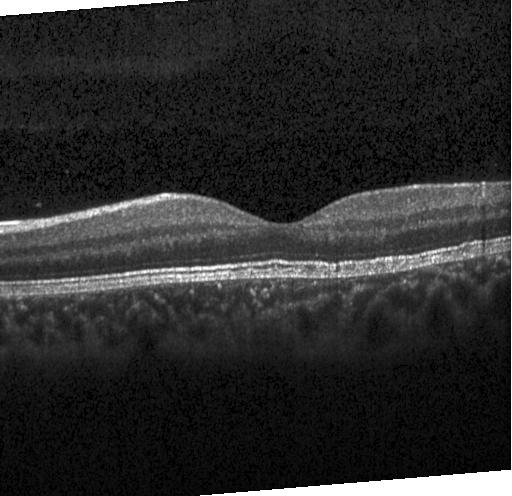 Macular scan · Heidelberg Spectralis · SD-OCT · OCT B-scan. Impression: no evidence of choroidal neovascularization, diabetic macular edema, or drusen.